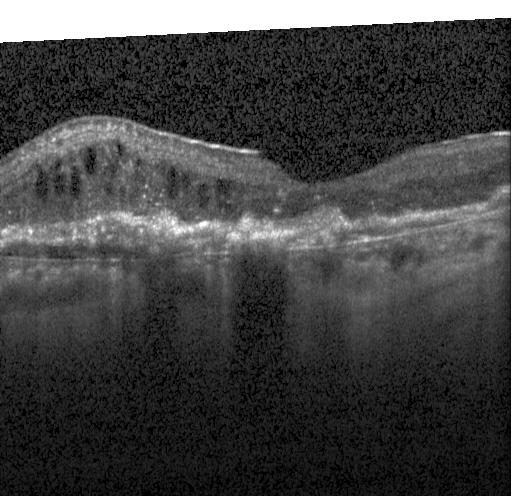

Heidelberg Spectralis OCT system; SD-OCT; OCT line scan
CNV.